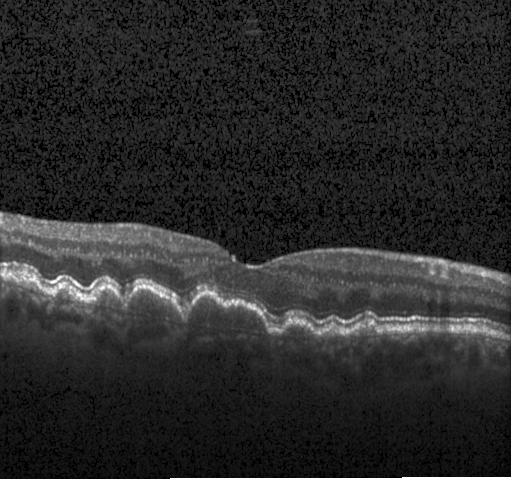 Dx: multiple drusen.